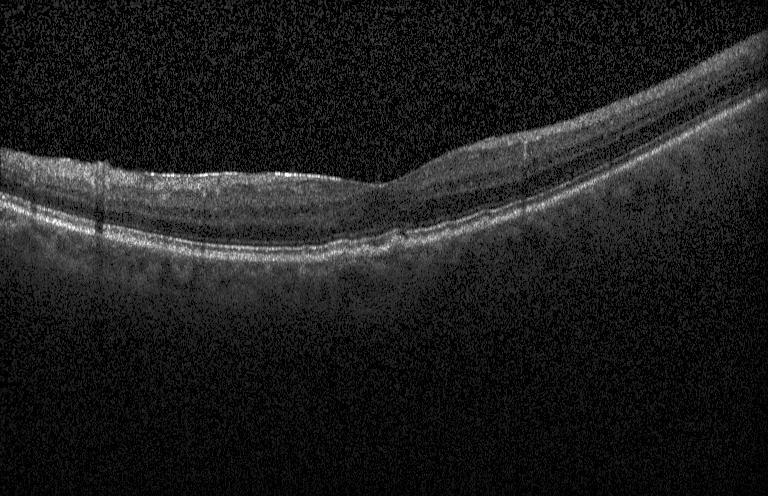

Finding: drusen.